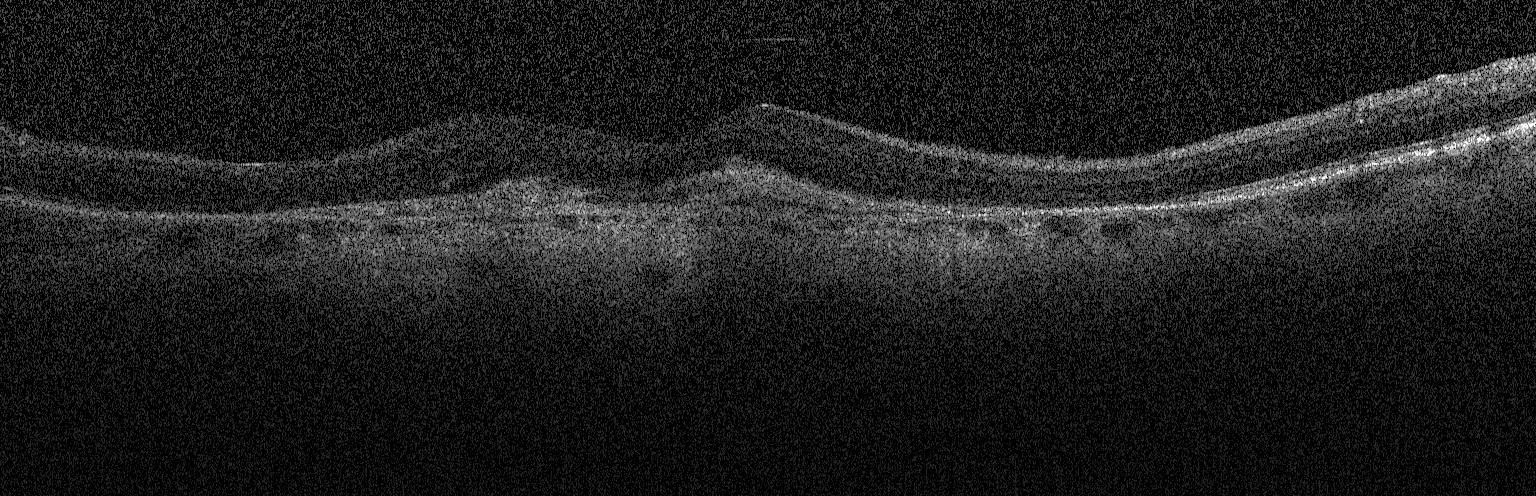
Centered on the fovea; spectral-domain optical coherence tomography; instrument: Heidelberg Spectralis; OCT line scan — This B-scan demonstrates choroidal neovascularization.